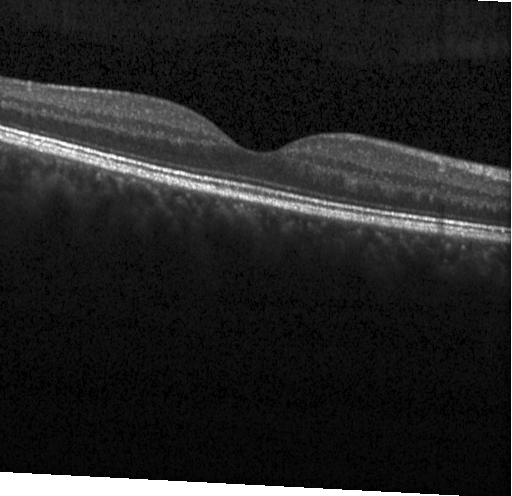
Spectral-domain OCT B-scan: no choroidal neovascularization, no diabetic macular edema, and no drusen.